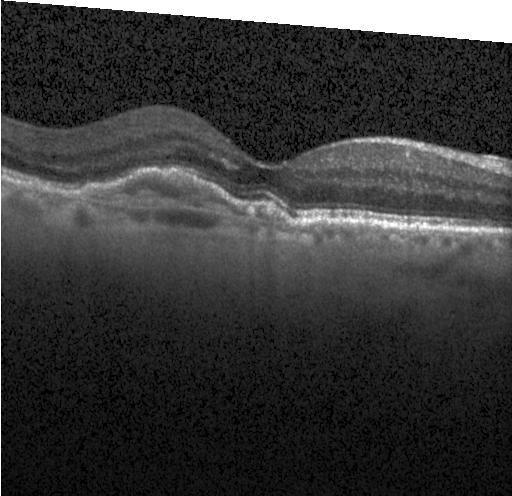 OCT line scan.
Diagnosis: a choroidal neovascular membrane.